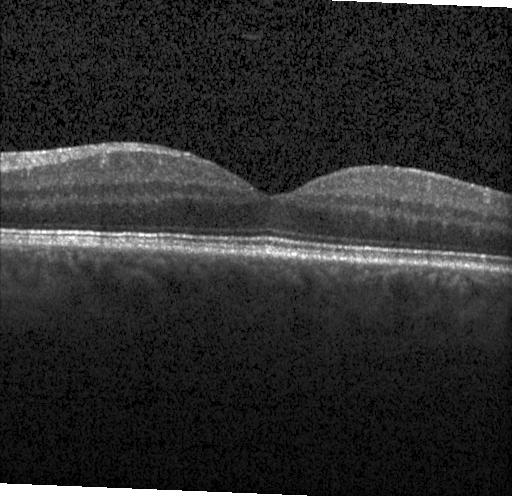

Dx: no choroidal neovascularization, no diabetic macular edema, and no drusen.